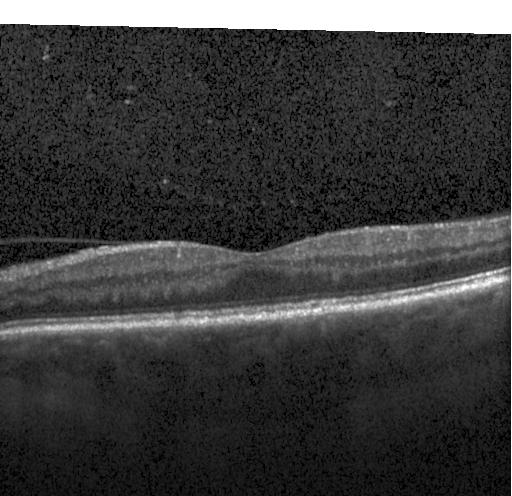 Spectral-domain optical coherence tomography, OCT line scan, acquired on a Heidelberg Spectralis
OCT finding: no choroidal neovascularization, diabetic macular edema, or drusen.